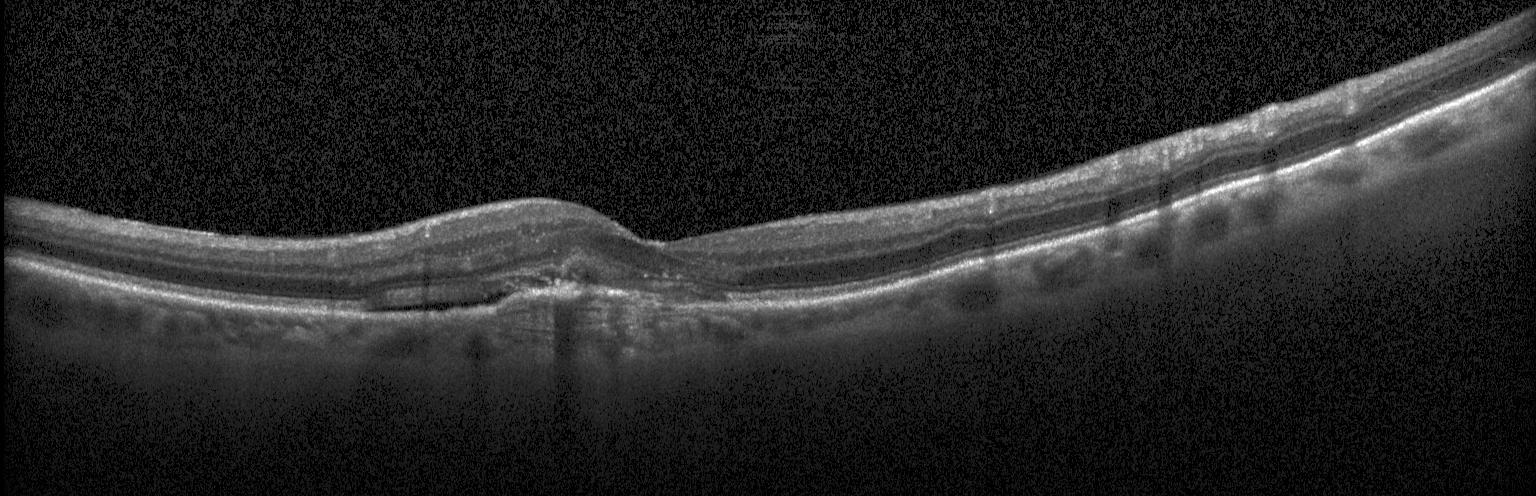

Assessment: choroidal neovascularization.